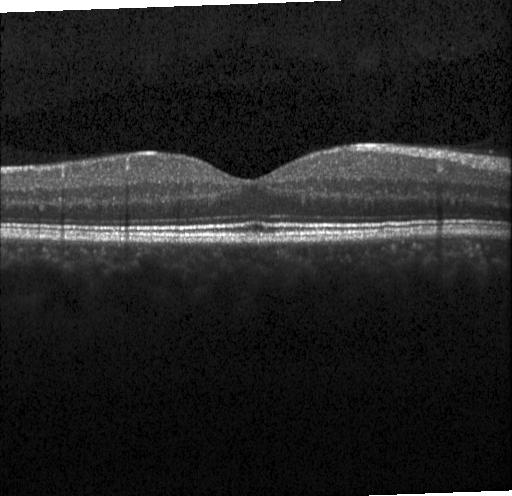 OCT B-scan · SD-OCT · Heidelberg Spectralis OCT system · centered on the fovea. Macular OCT: no CNV, DME, or drusen.